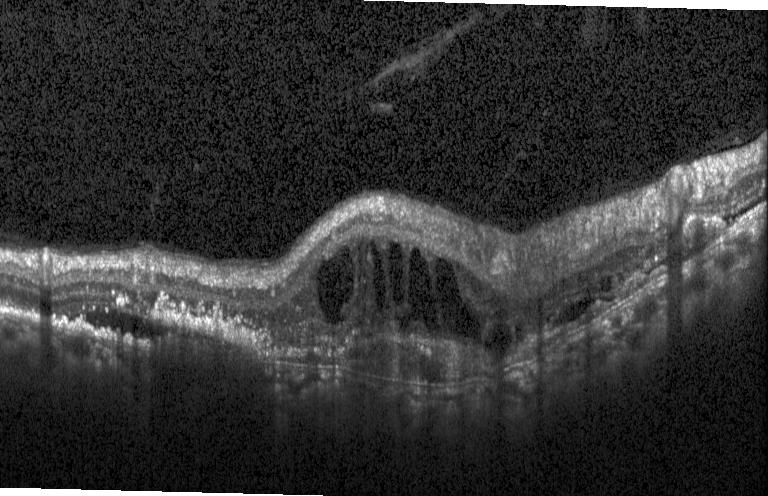

Macular OCT demonstrating a choroidal neovascular membrane.